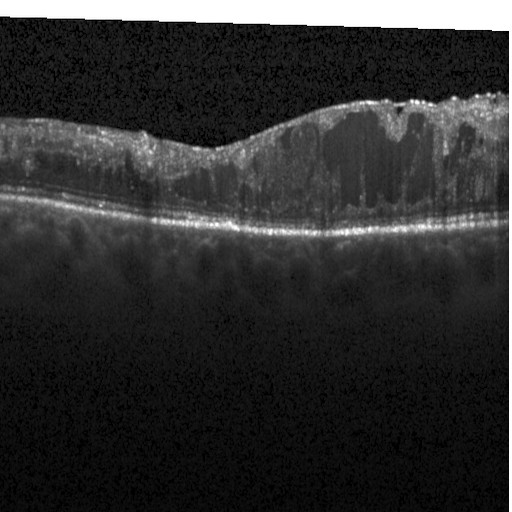

Optical coherence tomography scan — Macular OCT: diabetic macular edema (DME).